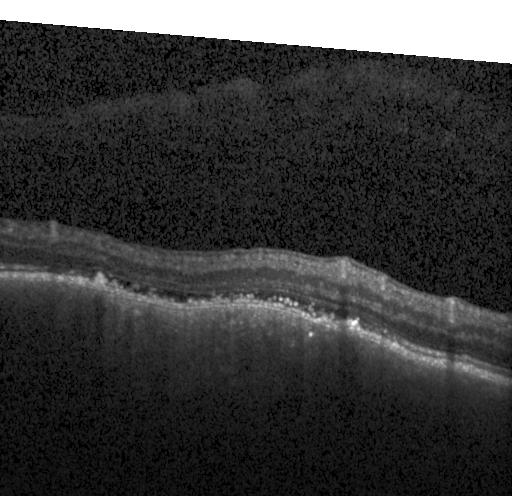 Dx: a choroidal neovascular membrane.